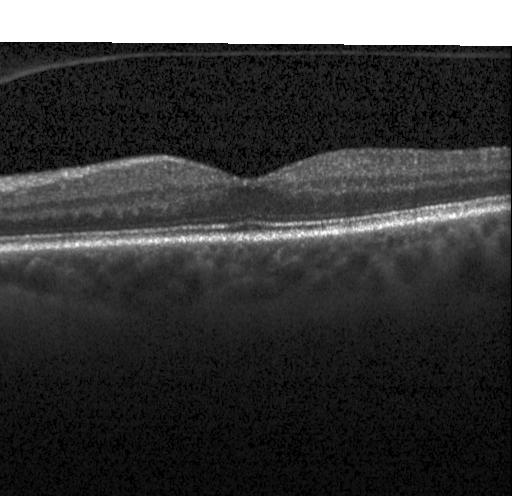

SD-OCT, Heidelberg Spectralis, retinal OCT B-scan, macular scan. Finding: no choroidal neovascularization, no diabetic macular edema, and no drusen.